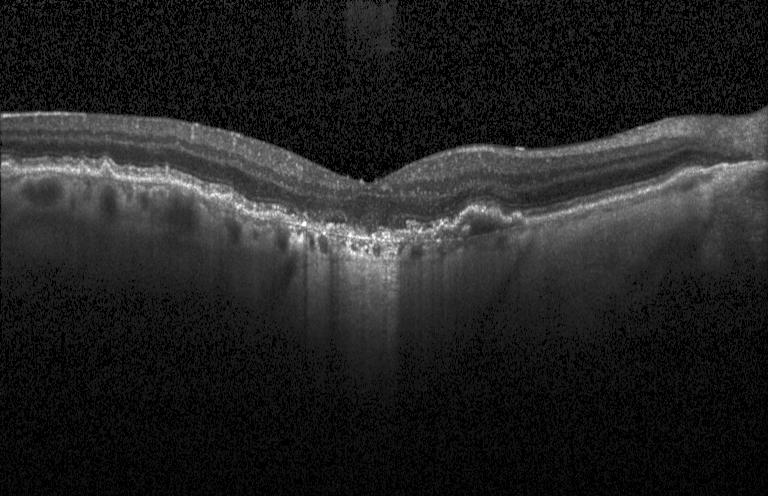
OCT scan showing CNV.